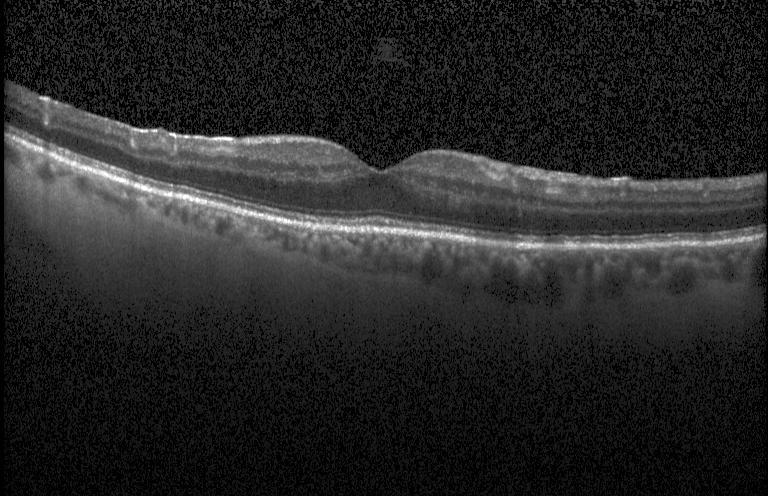 Instrument: Heidelberg Spectralis, SD-OCT, OCT line scan, fovea-centered. OCT finding: no choroidal neovascularization, diabetic macular edema, or drusen.